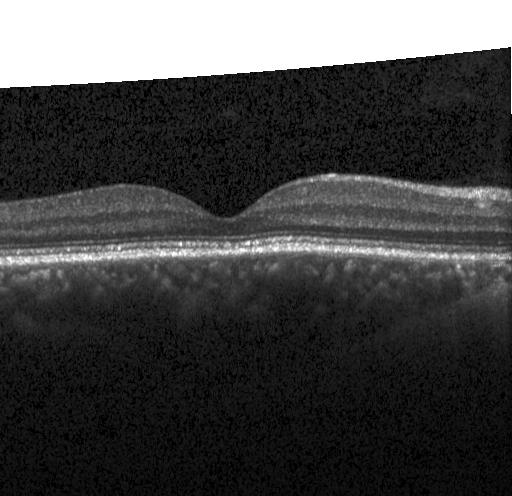

Heidelberg Spectralis, OCT B-scan, horizontal scan through the fovea — Impression: no evidence of choroidal neovascularization, diabetic macular edema, or drusen.